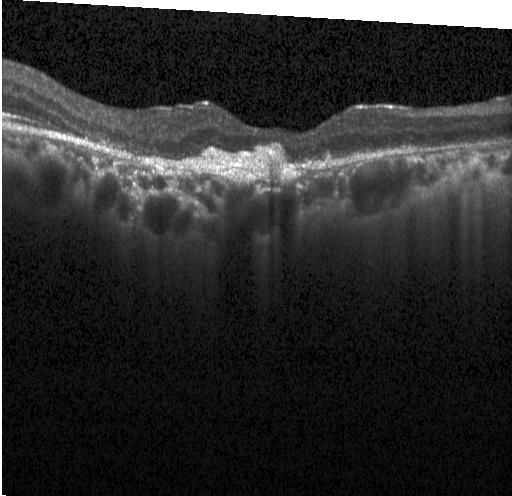

Dx: choroidal neovascularization (CNV).